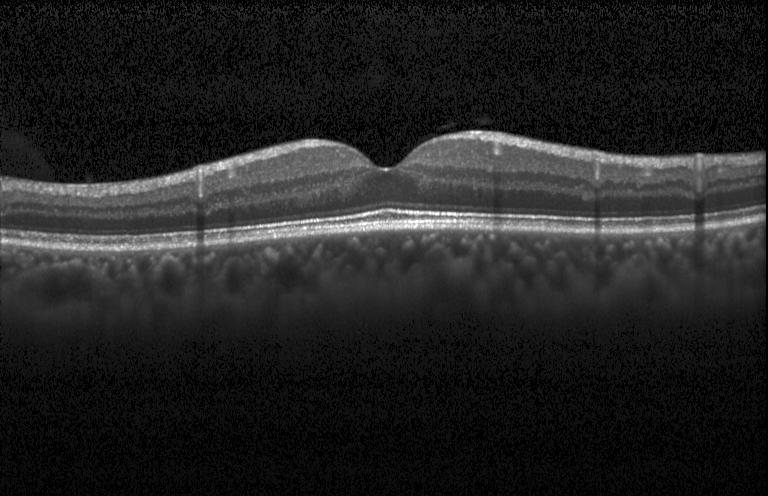 Spectral-domain OCT B-scan: no CNV, no DME, and no drusen.